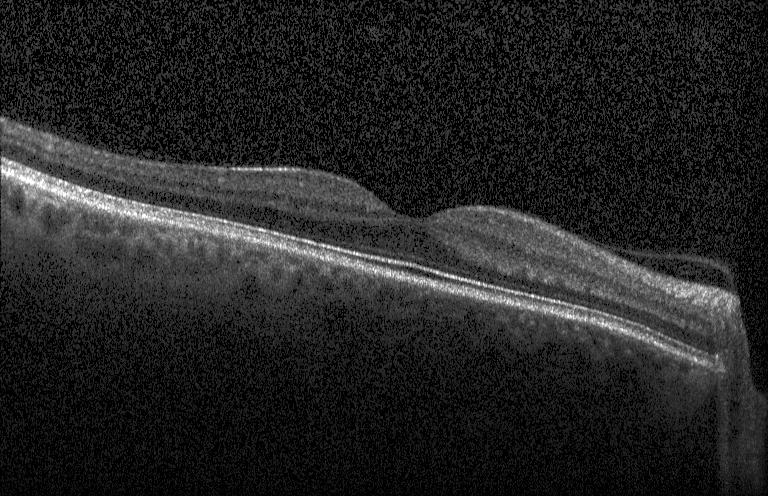 OCT B-scan. Instrument: Heidelberg Spectralis.
The scan shows no CNV, no DME, and no drusen.